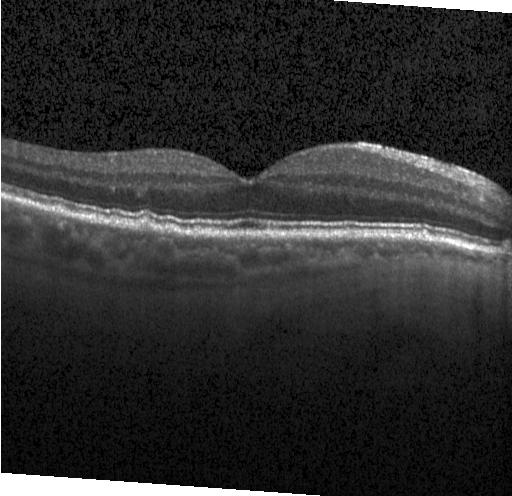
Spectral-domain optical coherence tomography; Heidelberg Spectralis; optical coherence tomography scan; fovea-centered — Finding: drusen.